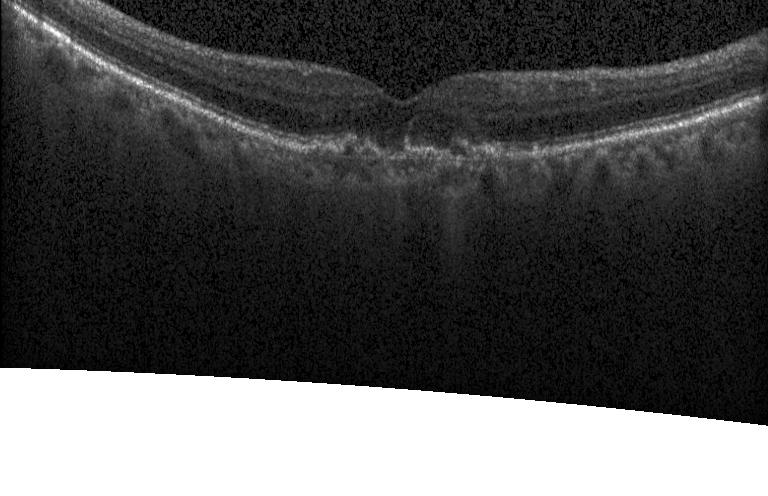 SD-OCT. Centered on the fovea. Instrument: Heidelberg Spectralis. OCT B-scan — Dx: a choroidal neovascular membrane.